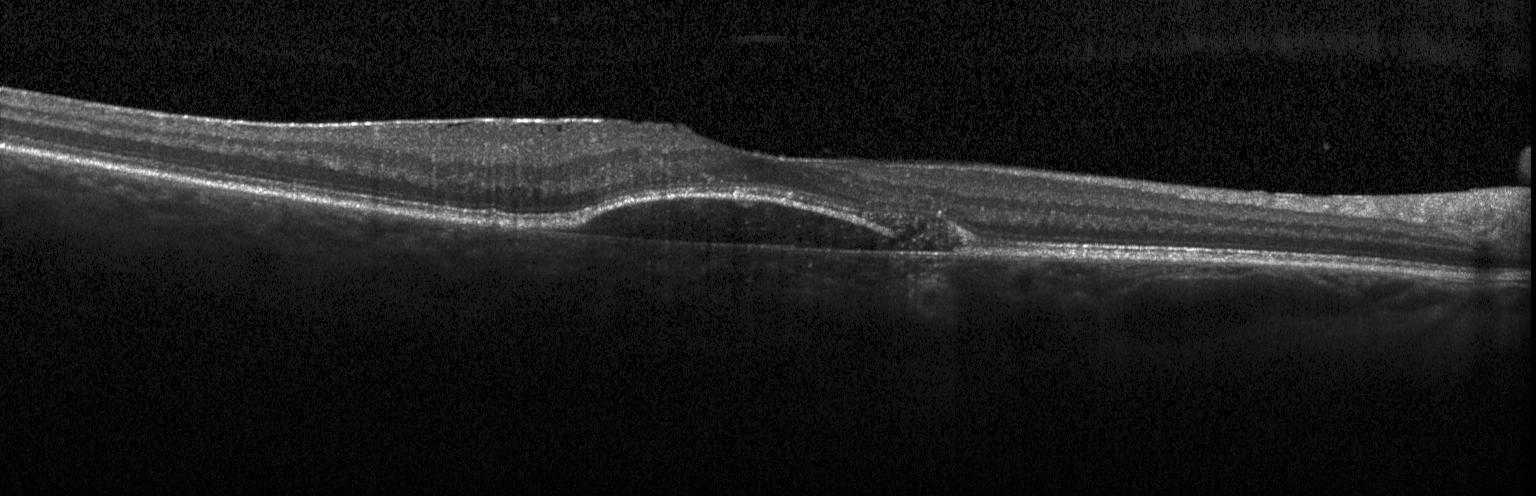 Heidelberg Spectralis OCT system; SD-OCT; horizontal scan through the fovea; retinal OCT cross-section
Choroidal neovascularization.